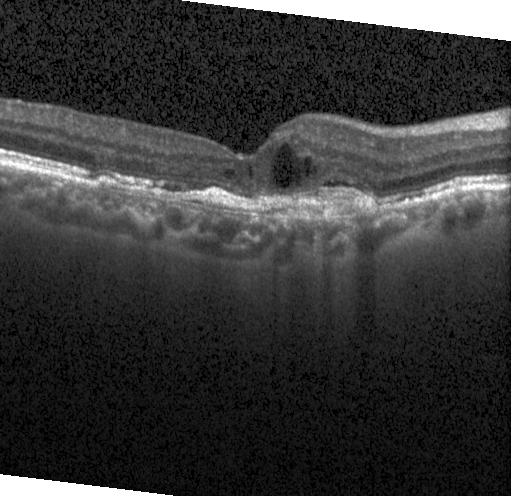
Centered on the fovea. Optical coherence tomography scan. Spectral-domain optical coherence tomography. A choroidal neovascular membrane.